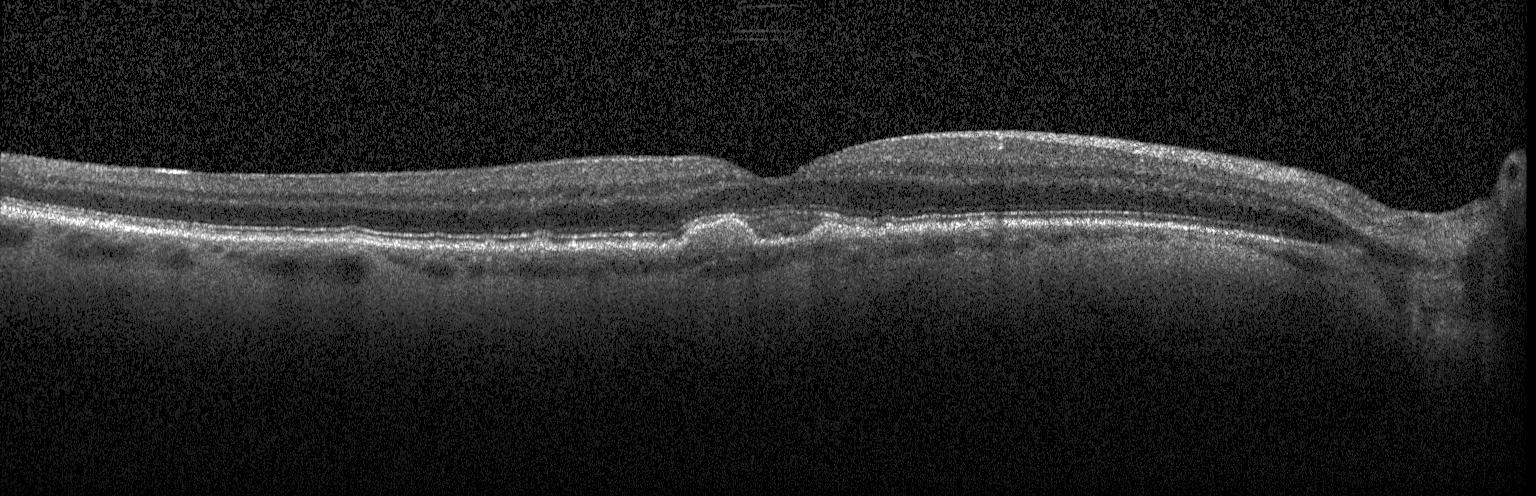 OCT line scan · SD-OCT · Heidelberg Spectralis · horizontal scan through the fovea — Finding: sub-RPE drusenoid deposits.